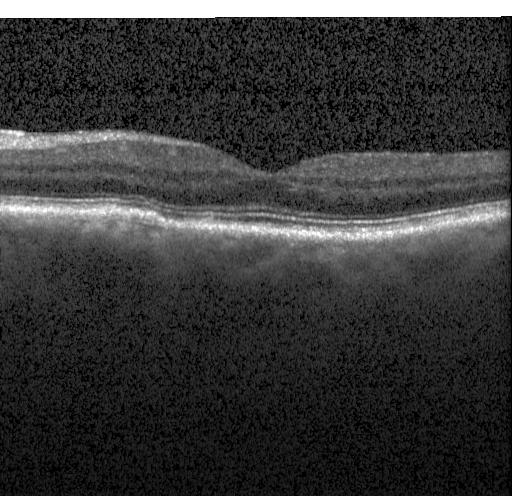

OCT line scan. Spectral-domain optical coherence tomography. Acquired on a Heidelberg Spectralis. Horizontal scan through the fovea. OCT finding: drusen.